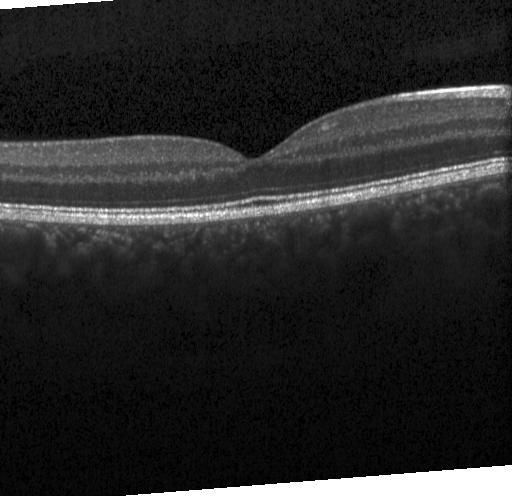
Impression: no choroidal neovascularization, no diabetic macular edema, and no drusen.